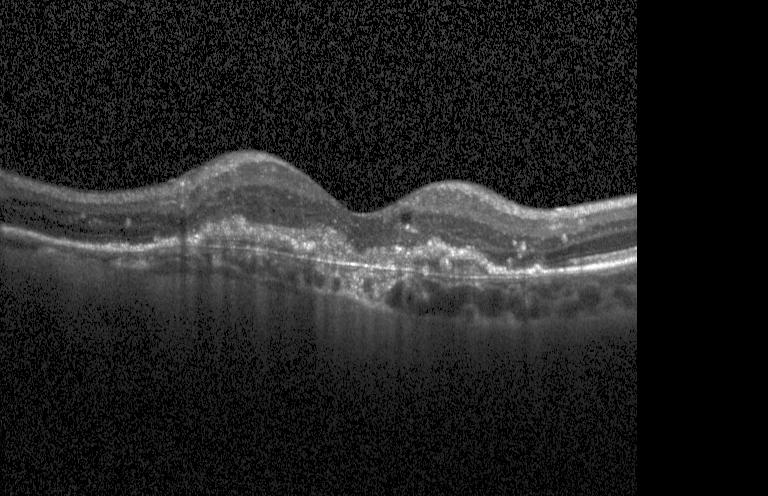

Impression: a choroidal neovascular membrane.